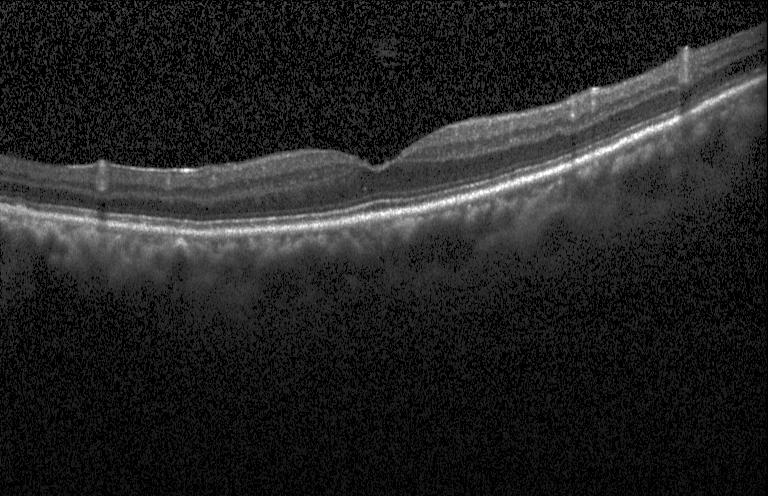 Optical coherence tomography B-scan, acquired on a Heidelberg Spectralis
OCT finding: no evidence of choroidal neovascularization, diabetic macular edema, or drusen.